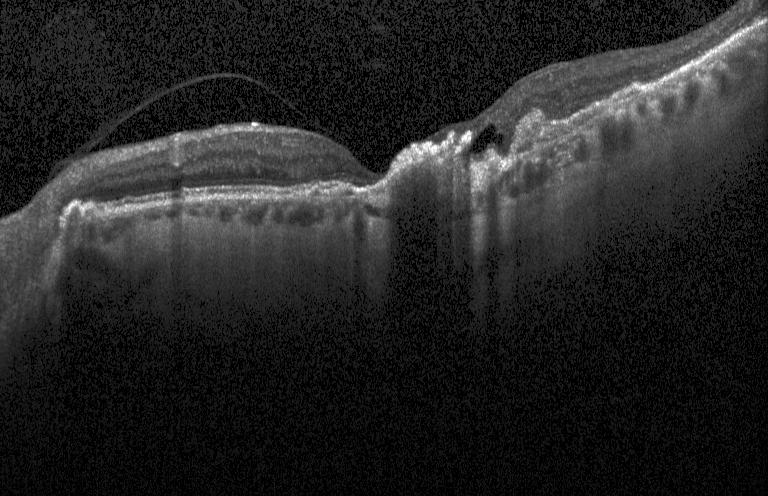 Acquired on a Heidelberg Spectralis; spectral-domain OCT; horizontal scan through the fovea; optical coherence tomography B-scan. Dx: a choroidal neovascular membrane.